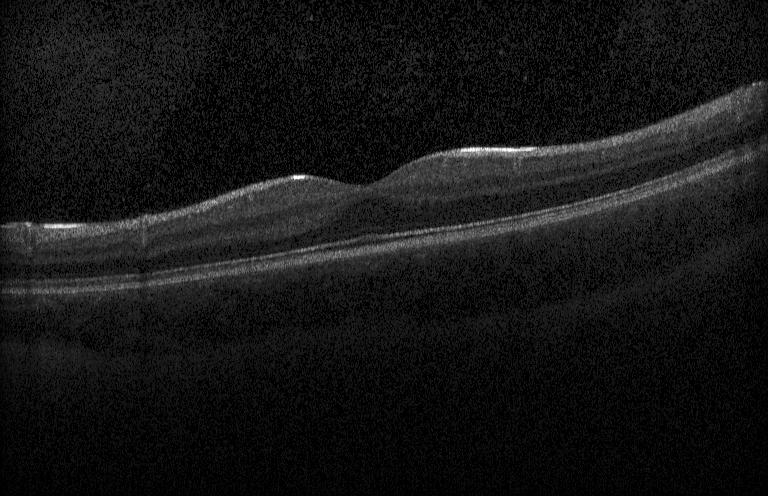 Assessment: no evidence of CNV, DME, or drusen.